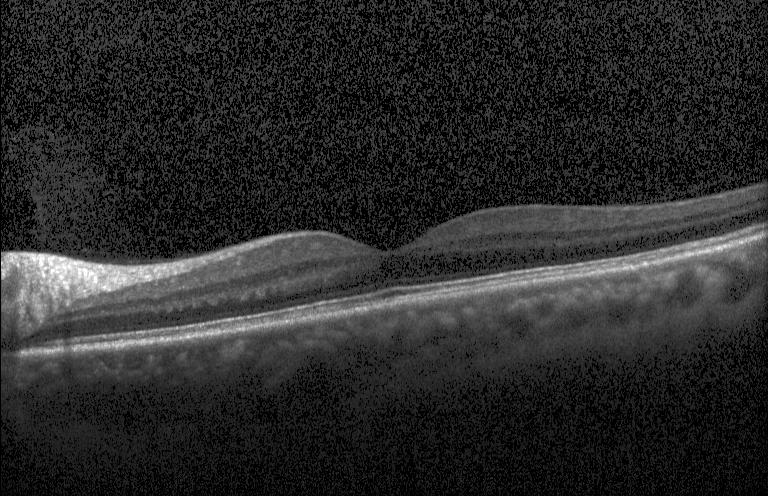 Optical coherence tomography B-scan, centered on the fovea.
Impression: no choroidal neovascularization, no diabetic macular edema, and no drusen.